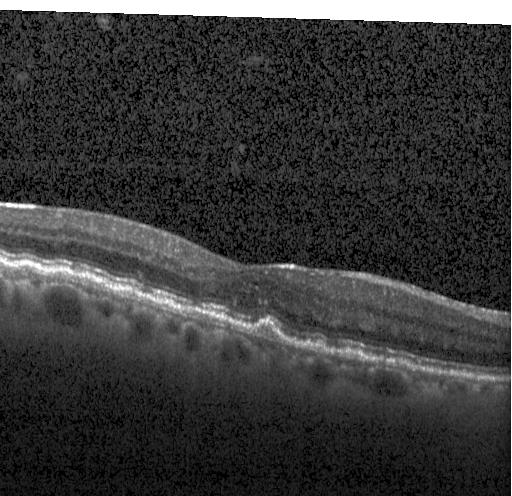
Sub-RPE drusenoid deposits.